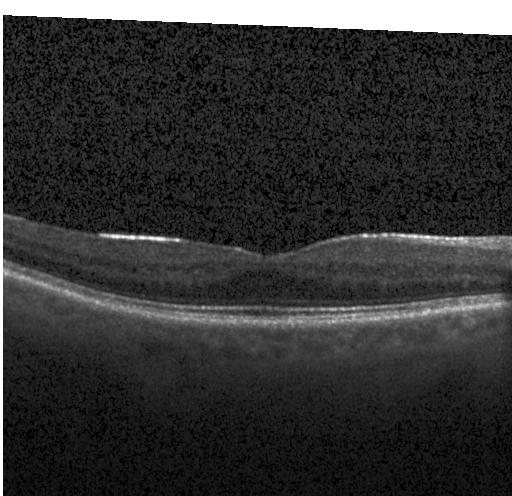

Retinal OCT cross-section showing no choroidal neovascularization, no diabetic macular edema, and no drusen.